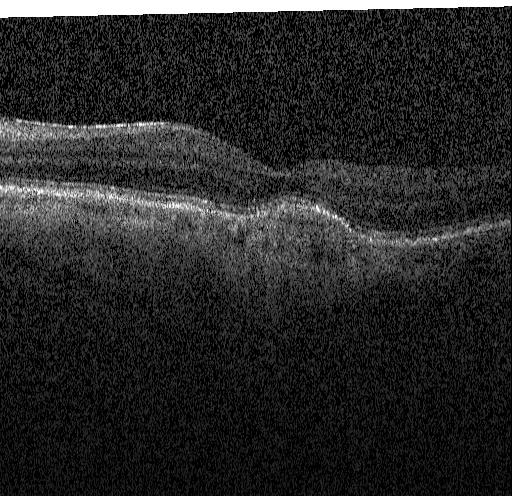 Heidelberg Spectralis OCT system; spectral-domain OCT; OCT line scan; through the macula — The scan shows choroidal neovascularization.